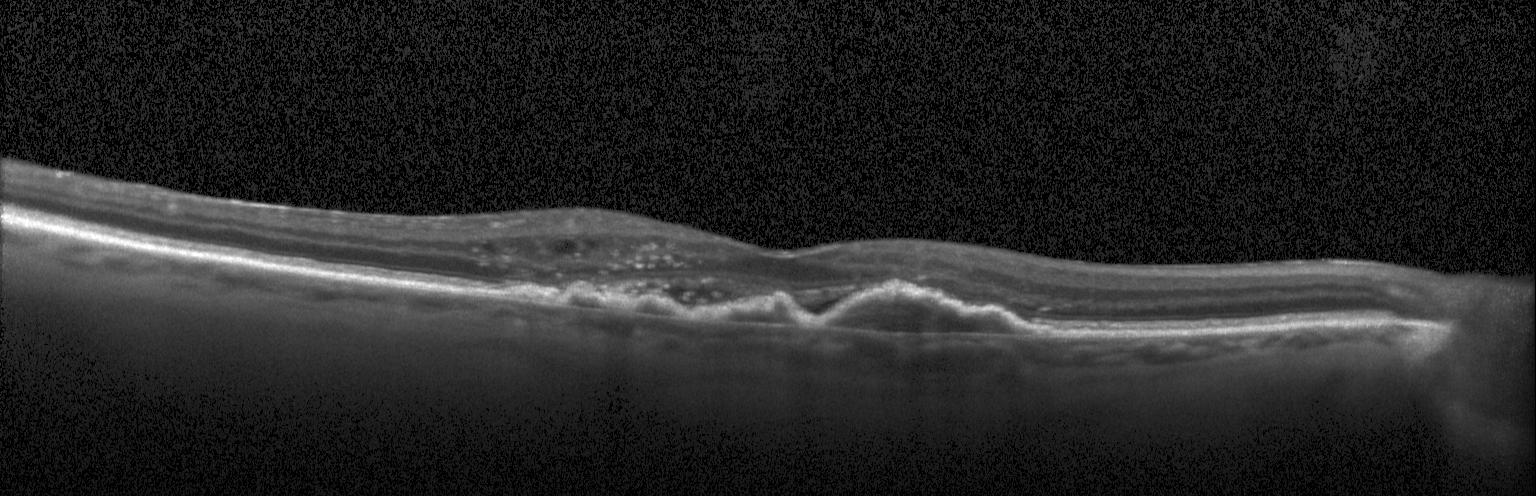 OCT finding: a choroidal neovascular membrane.